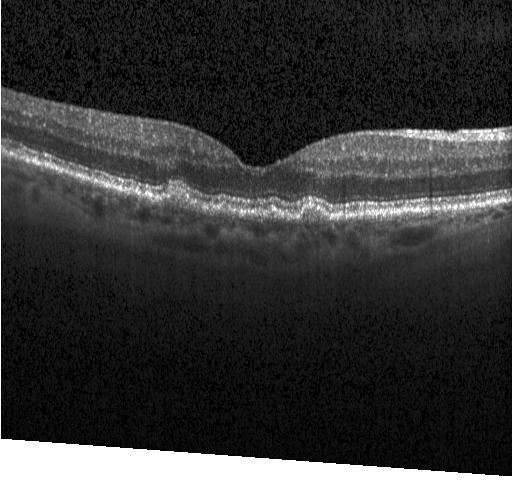 Multiple drusen.